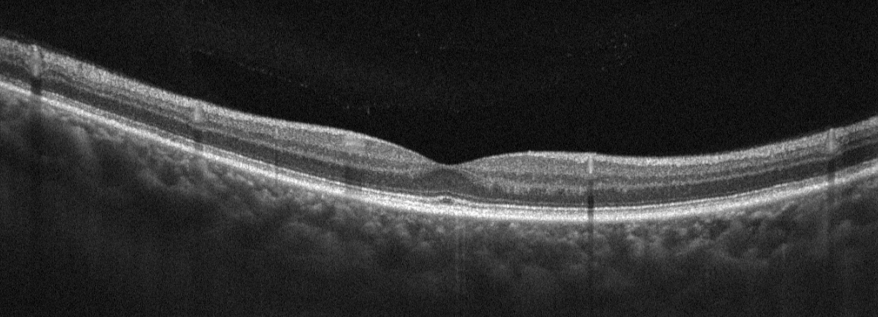
Macular OCT: no evidence of AMD, DME, ERM, RAO, RVO, or VID.